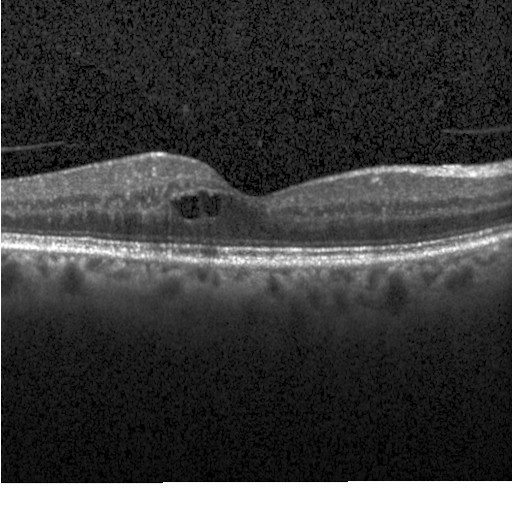
Spectral-domain OCT B-scan: diabetic macular edema.